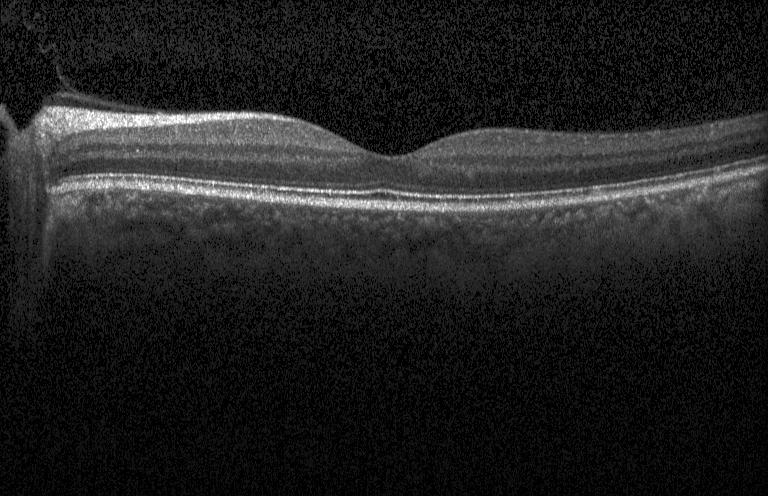
Retinal OCT B-scan. Acquired on a Heidelberg Spectralis. Centered on the fovea
Impression: no evidence of choroidal neovascularization, diabetic macular edema, or drusen.